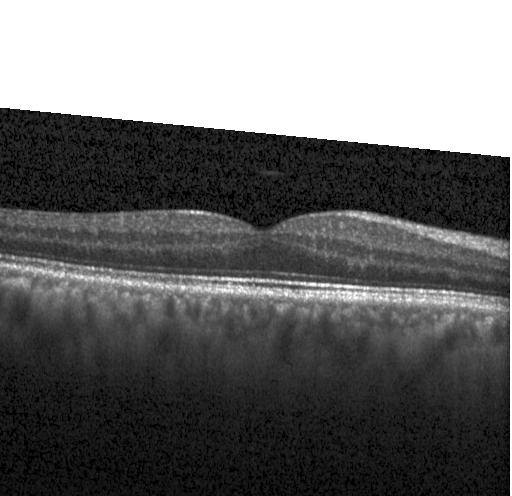
Fovea-centered, spectral-domain optical coherence tomography, instrument: Heidelberg Spectralis, retinal OCT cross-section.
Finding: no choroidal neovascularization, no diabetic macular edema, and no drusen.